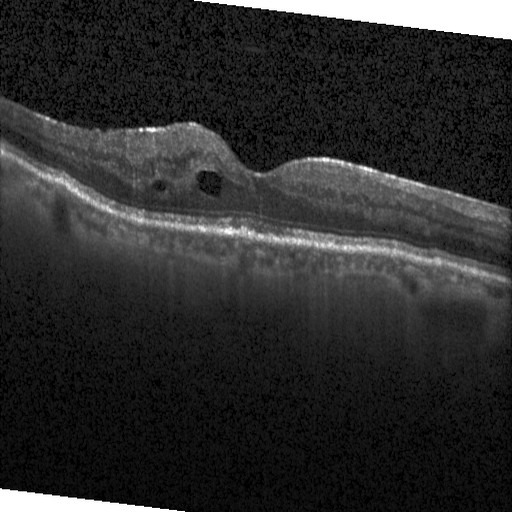
Spectral-domain OCT; OCT B-scan
Finding: diabetic macular edema.